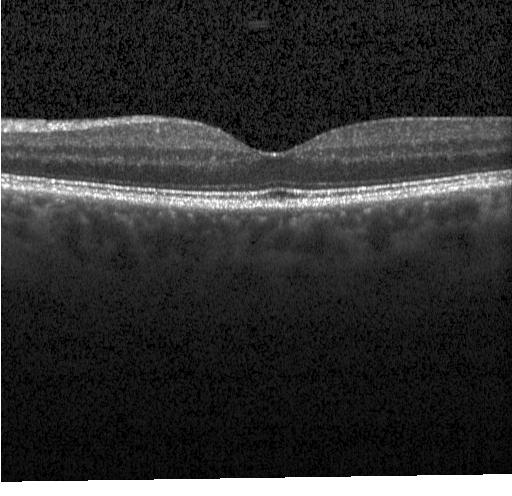

Dx: no choroidal neovascularization, diabetic macular edema, or drusen.